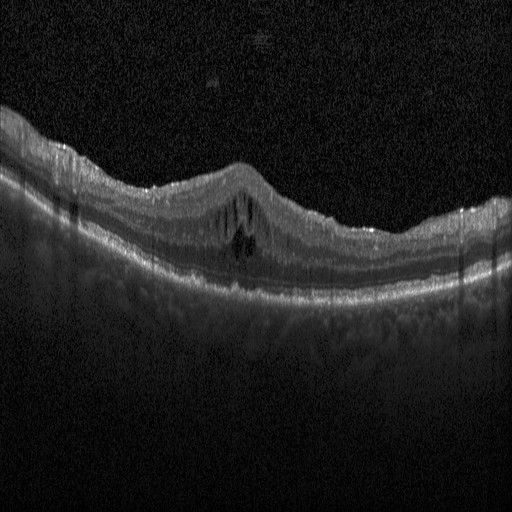
OCT scan showing diabetic macular edema.